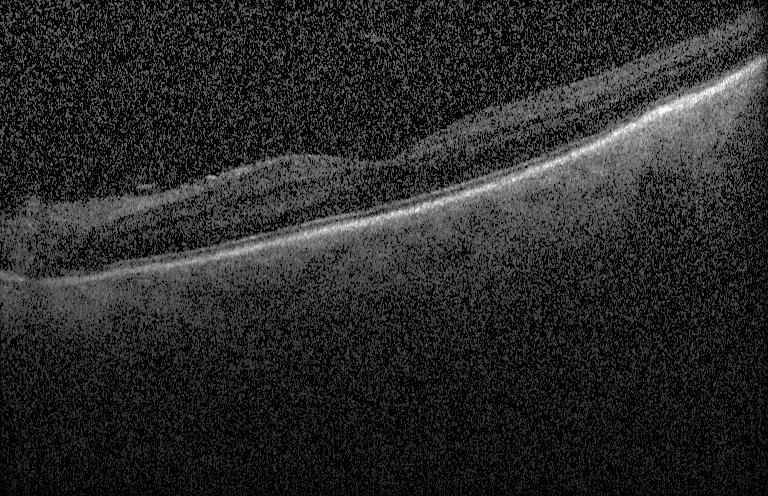
Retinal OCT B-scan — Impression: no evidence of CNV, DME, or drusen.